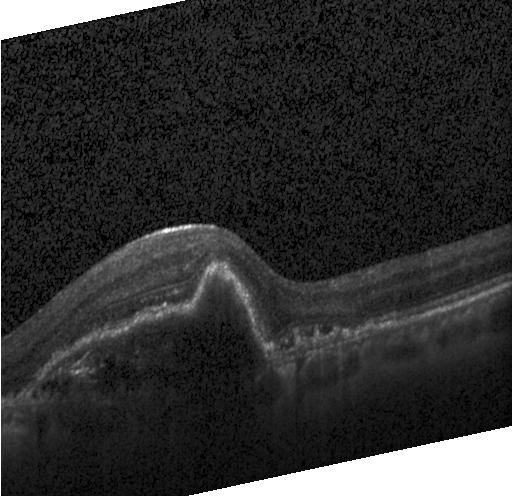

Optical coherence tomography B-scan · Heidelberg Spectralis OCT system.
Macular OCT: choroidal neovascularization.